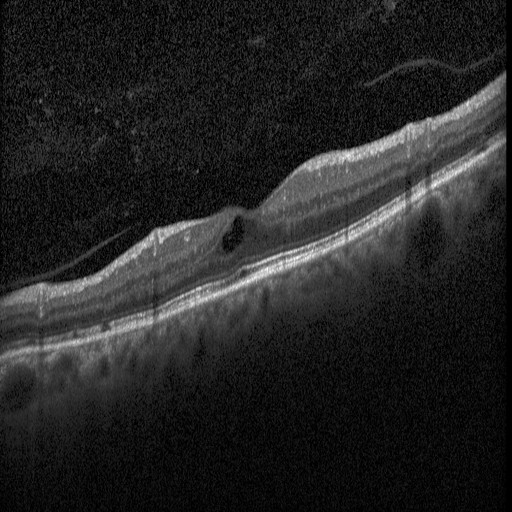 Through the macula · spectral-domain OCT · Heidelberg Spectralis · optical coherence tomography B-scan
Finding: DME.